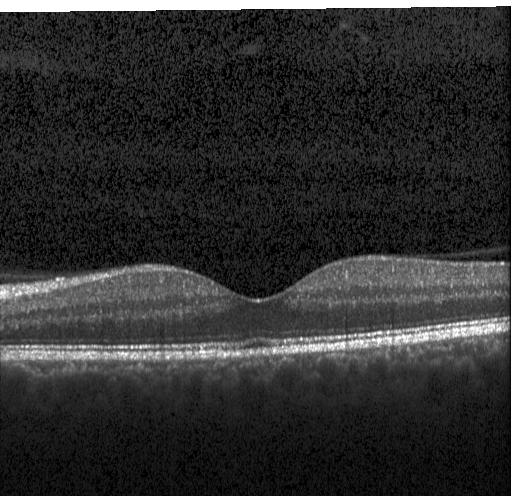

Optical coherence tomography B-scan
Assessment: no CNV, no DME, and no drusen.